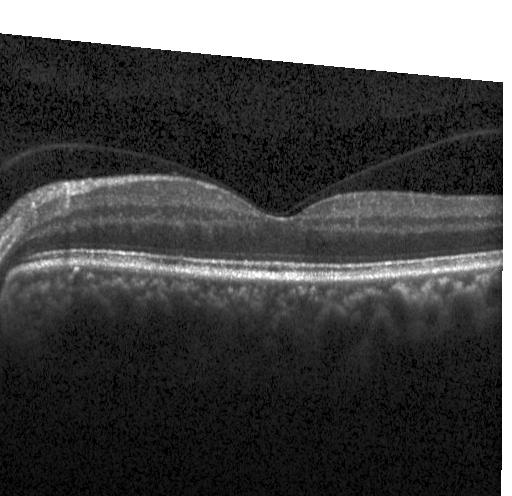

Instrument: Heidelberg Spectralis. Optical coherence tomography B-scan. Centered on the fovea. Spectral-domain optical coherence tomography.
This B-scan demonstrates neither choroidal neovascularization, diabetic macular edema, nor drusen.